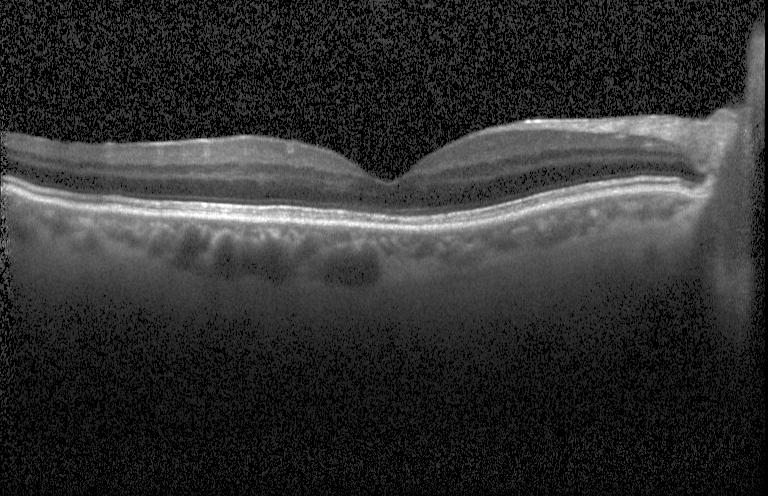
Macular scan. Retinal OCT cross-section. SD-OCT
Diagnosis: no choroidal neovascularization, diabetic macular edema, or drusen.